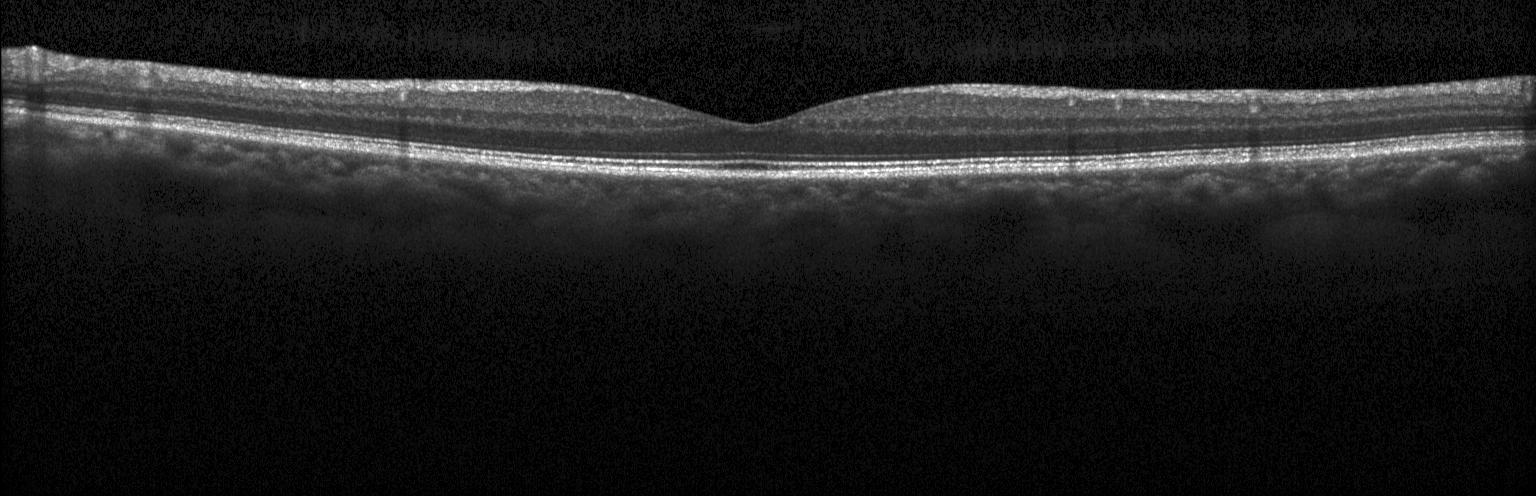
Retinal OCT cross-section showing no choroidal neovascularization, no diabetic macular edema, and no drusen.